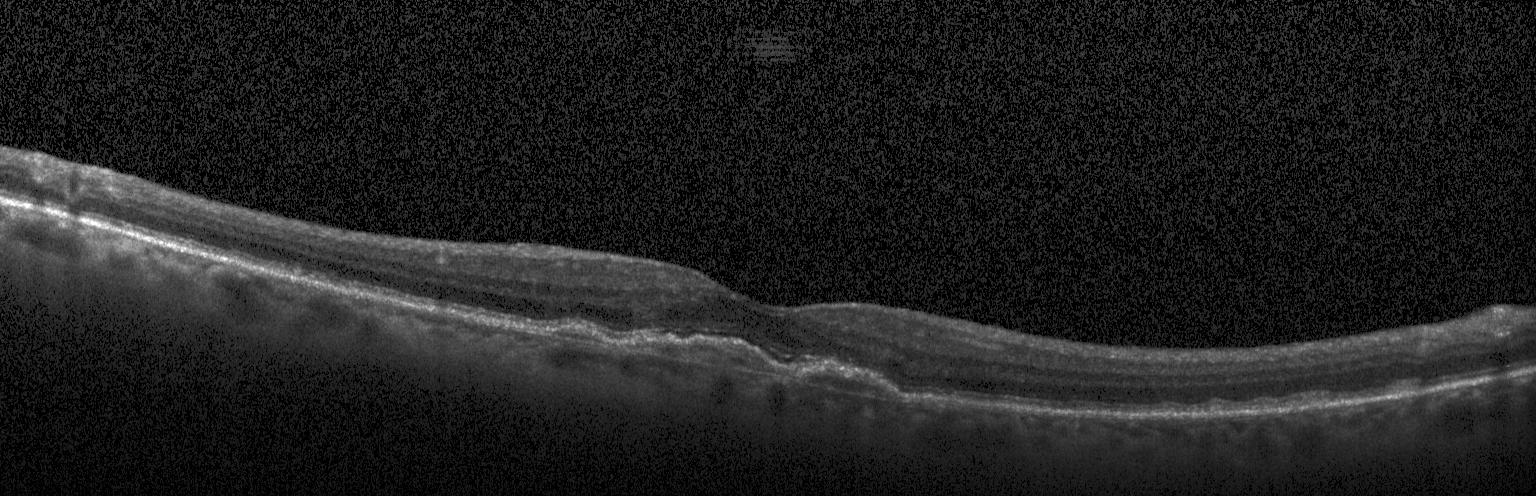 Dx: choroidal neovascularization.